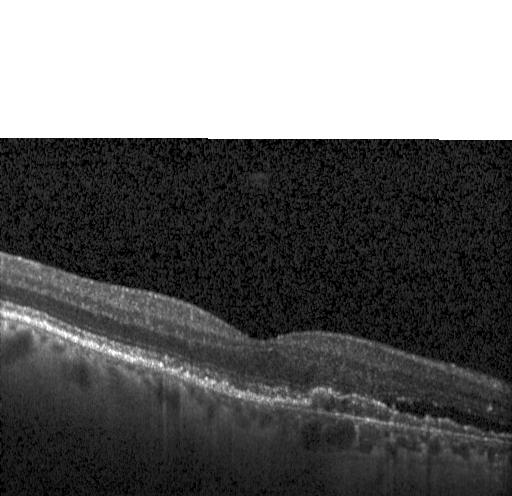

OCT line scan; horizontal scan through the fovea; SD-OCT. Finding: a choroidal neovascular membrane.